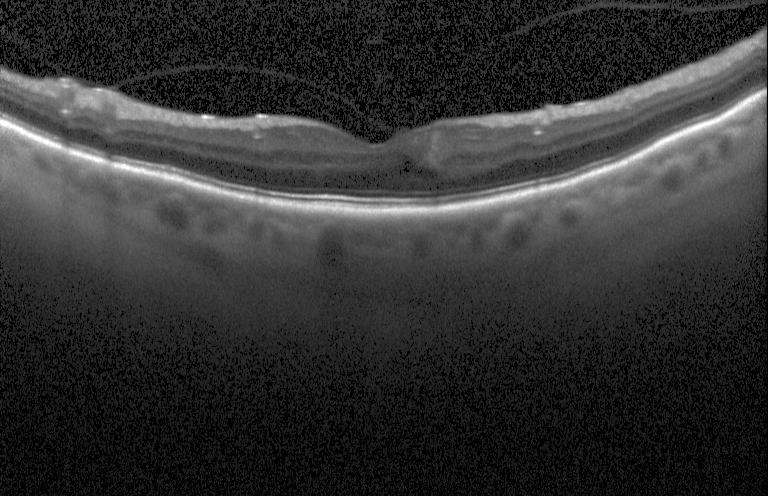 Centered on the fovea. Heidelberg Spectralis. Retinal OCT B-scan. SD-OCT. Macular OCT: diabetic macular edema.